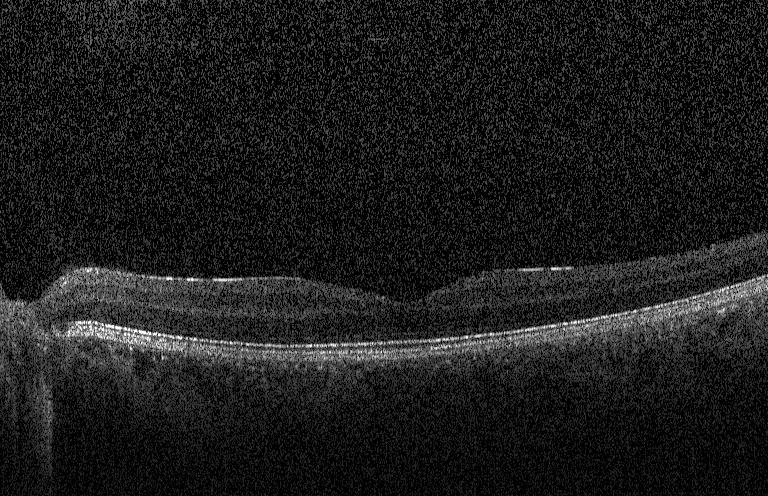
Spectral-domain optical coherence tomography; retinal OCT cross-section; Heidelberg Spectralis. Impression: neither choroidal neovascularization, diabetic macular edema, nor drusen.